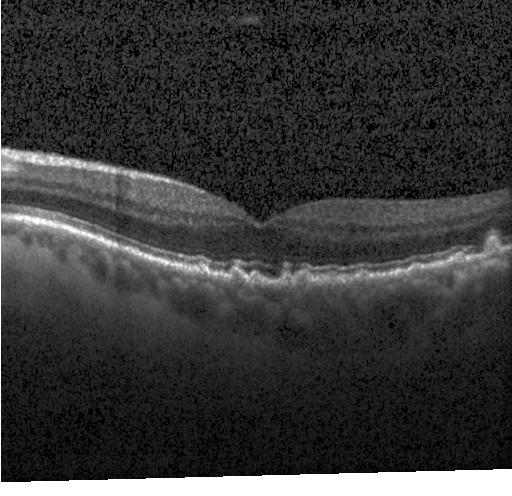
Retinal OCT cross-section. Spectral-domain OCT — OCT finding: multiple drusen.